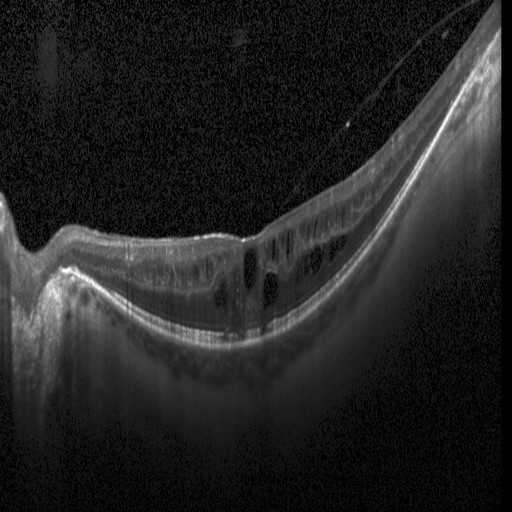

OCT line scan, spectral-domain OCT, Heidelberg Spectralis OCT system.
DME.